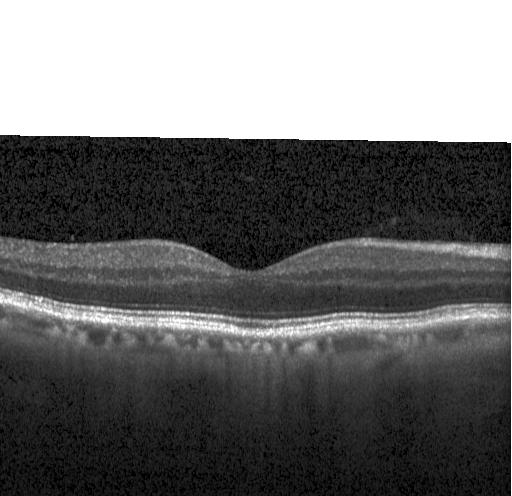
Instrument: Heidelberg Spectralis; retinal OCT B-scan; spectral-domain optical coherence tomography; fovea-centered
Diagnosis: neither choroidal neovascularization, diabetic macular edema, nor drusen.